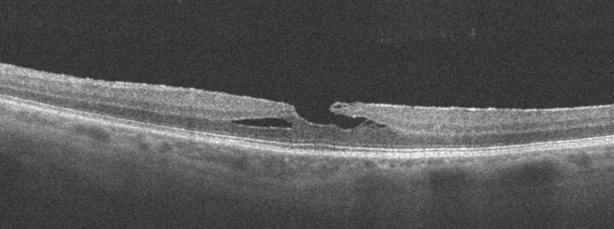

OCT scan showing vitreomacular interface disease.